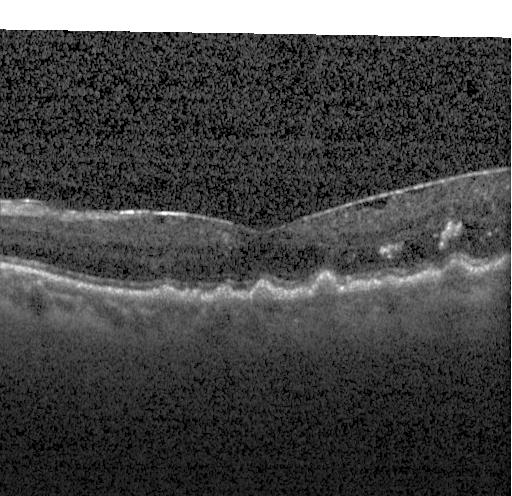
Macular OCT demonstrating drusen.